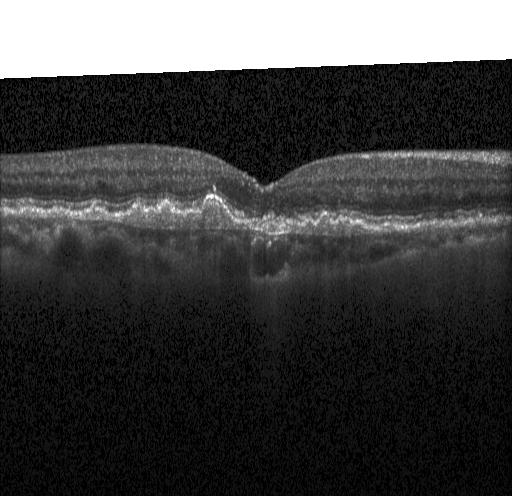
Through the macula, OCT line scan — Impression: choroidal neovascularization.